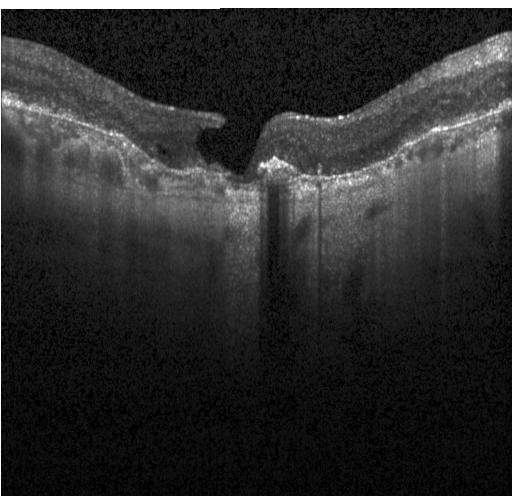

Spectral-domain OCT B-scan: CNV.